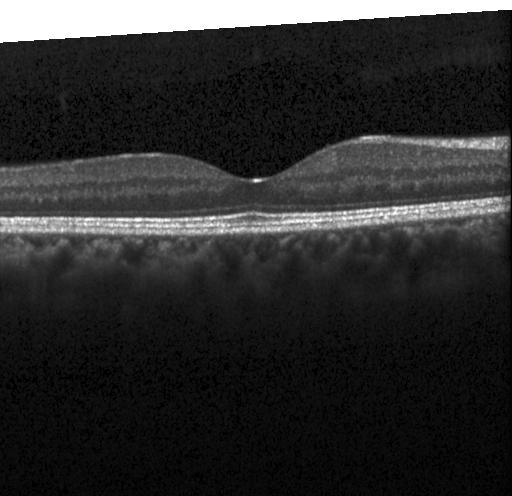 OCT finding: no evidence of choroidal neovascularization, diabetic macular edema, or drusen.